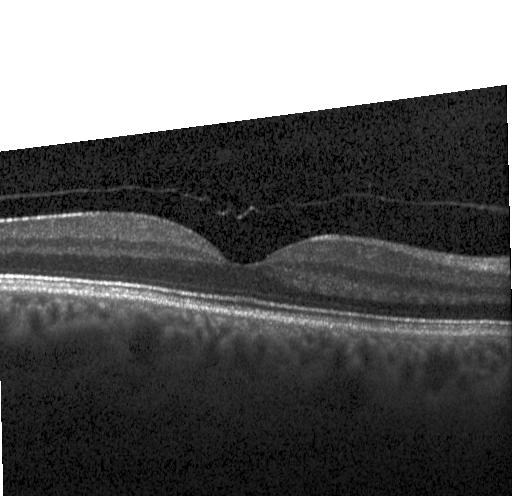
Macular OCT: no choroidal neovascularization, no diabetic macular edema, and no drusen.